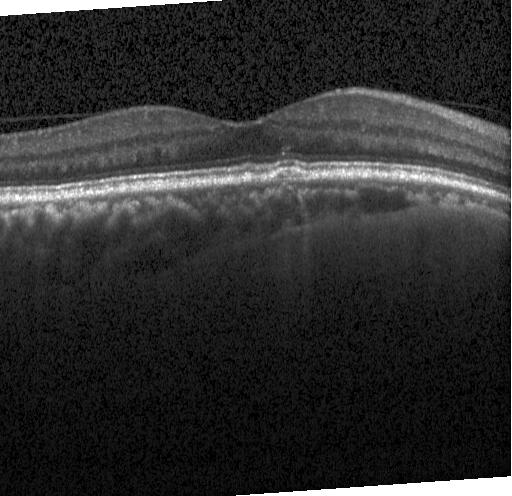
Retinal OCT cross-section showing multiple drusen.